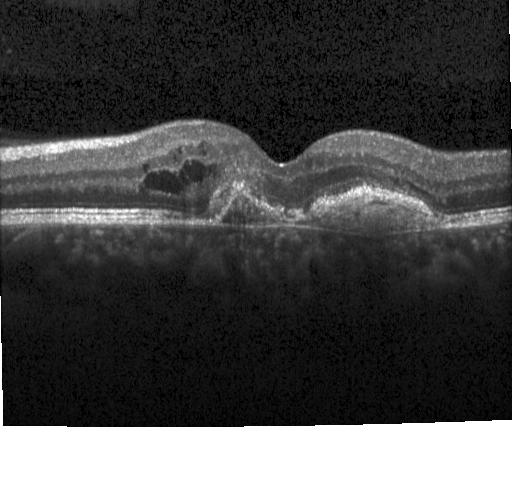
OCT line scan. Diagnosis: CNV.